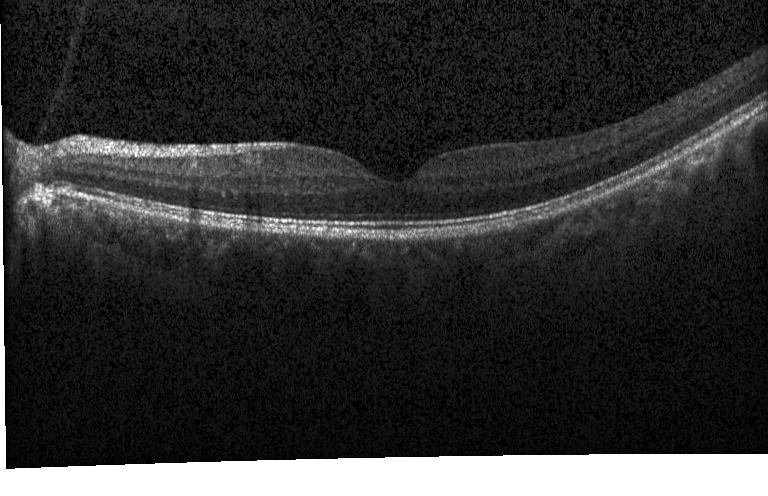 Diagnosis: no evidence of choroidal neovascularization, diabetic macular edema, or drusen.